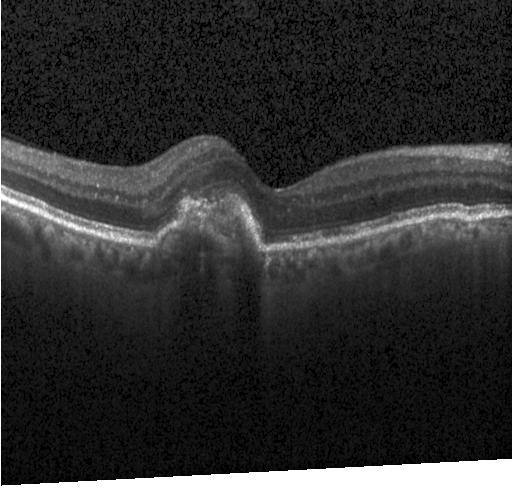

Impression: CNV.